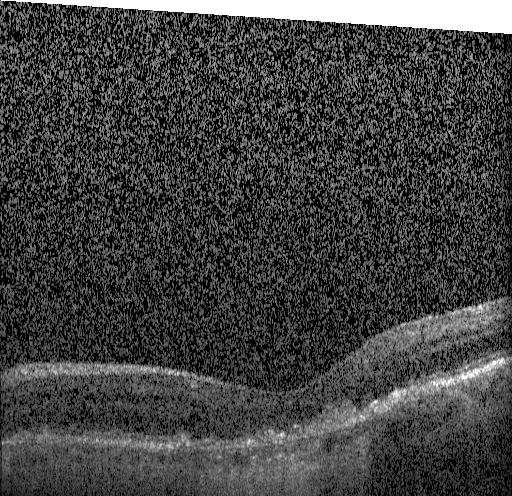
Retinal OCT cross-section showing CNV.